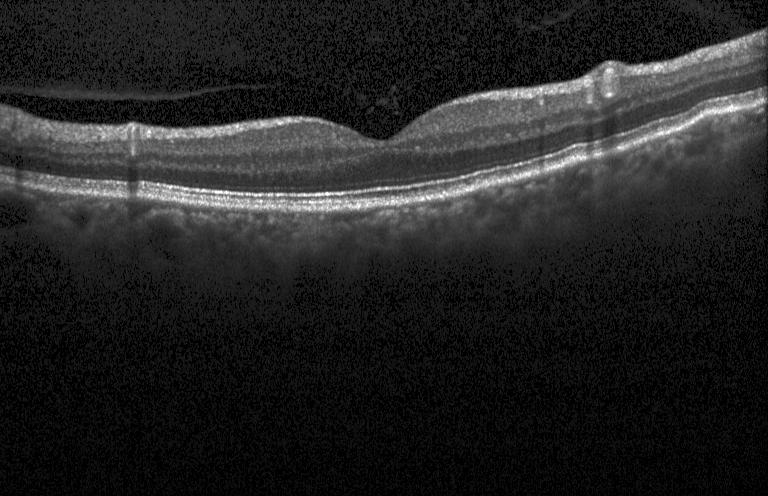

OCT B-scan; Heidelberg Spectralis OCT system; spectral-domain optical coherence tomography.
Diagnosis: no choroidal neovascularization, no diabetic macular edema, and no drusen.